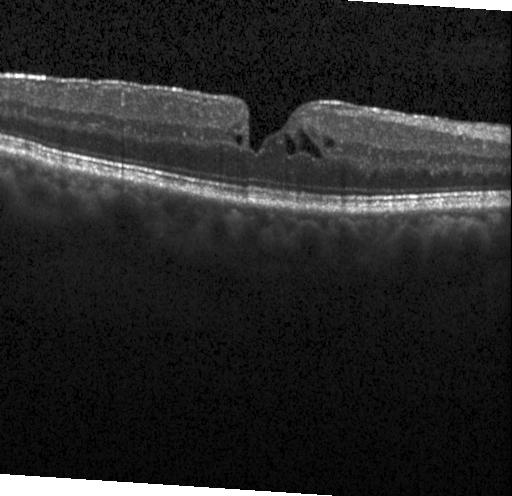 Instrument: Heidelberg Spectralis. Optical coherence tomography B-scan.
Diagnosis: diabetic macular edema (DME).